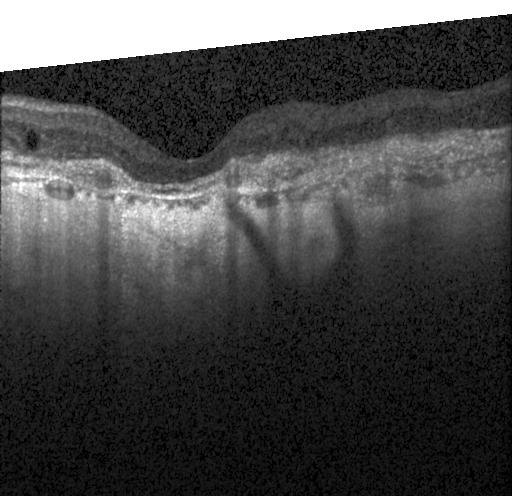
Through the macula; optical coherence tomography B-scan.
A choroidal neovascular membrane.